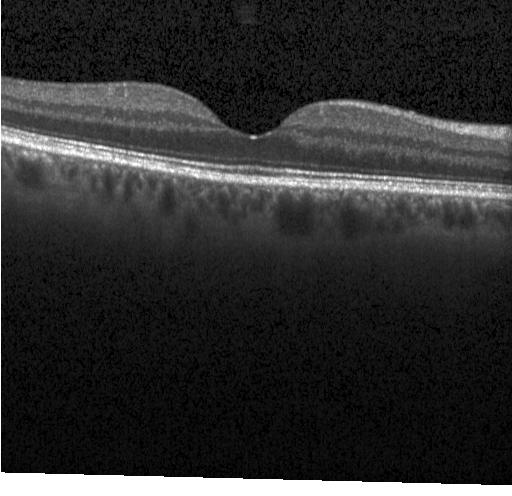

Macular OCT: neither choroidal neovascularization, diabetic macular edema, nor drusen.